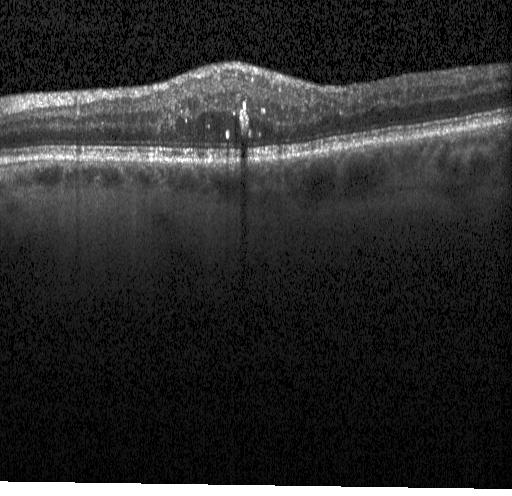

Diabetic macular edema.